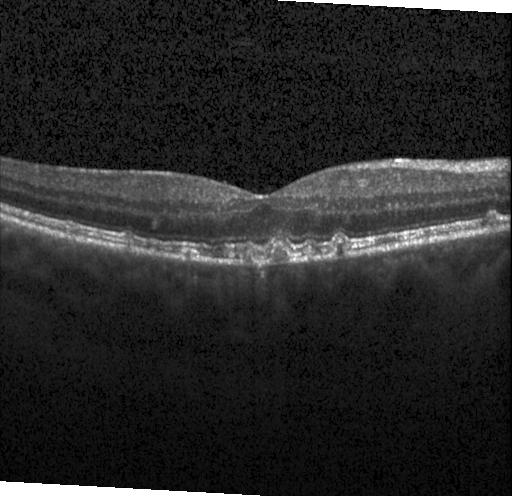 Retinal OCT B-scan; macular scan; Heidelberg Spectralis OCT system.
Finding: multiple drusen.